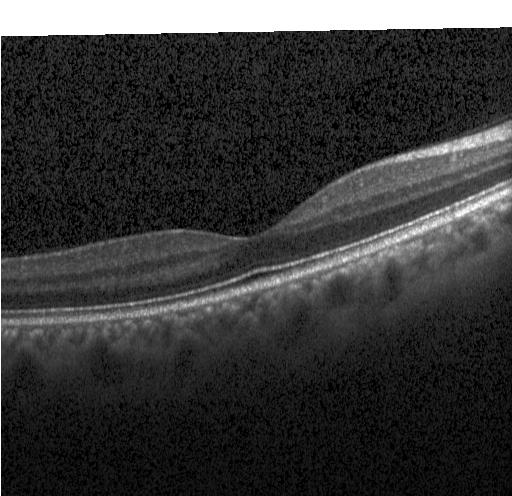 OCT finding: no choroidal neovascularization, diabetic macular edema, or drusen.